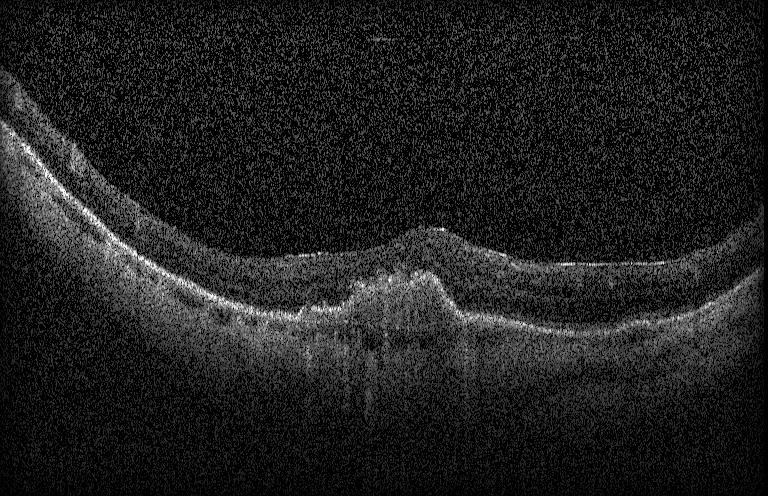 Retinal OCT cross-section — Finding: a choroidal neovascular membrane.